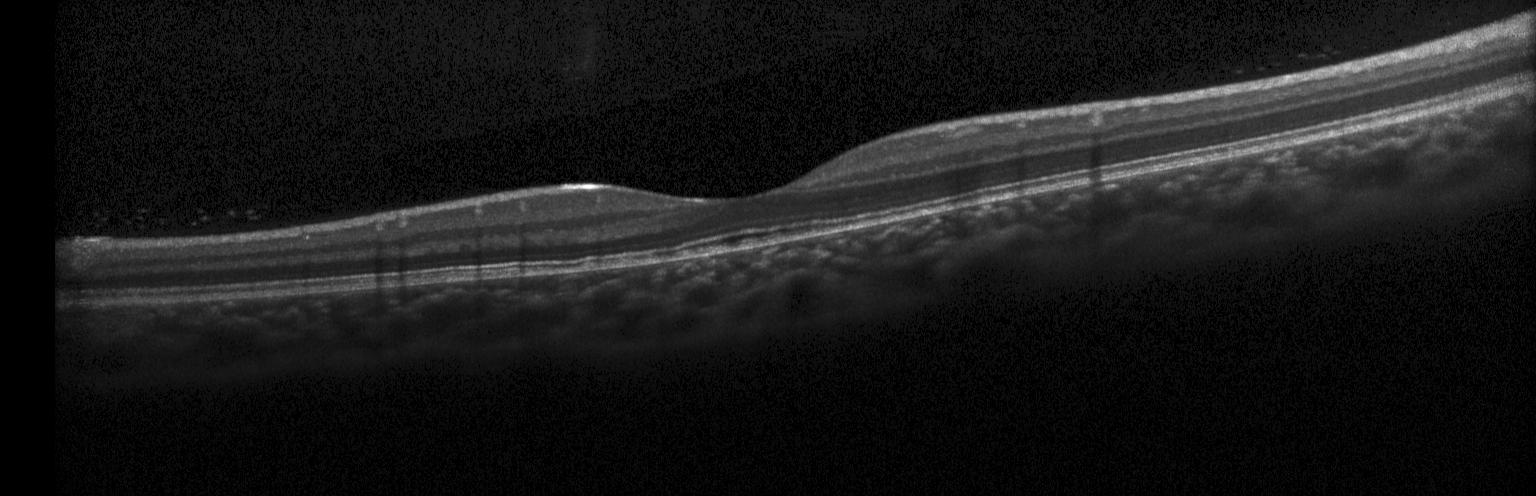

Horizontal scan through the fovea. Optical coherence tomography scan. Heidelberg Spectralis
Finding: neither choroidal neovascularization, diabetic macular edema, nor drusen.